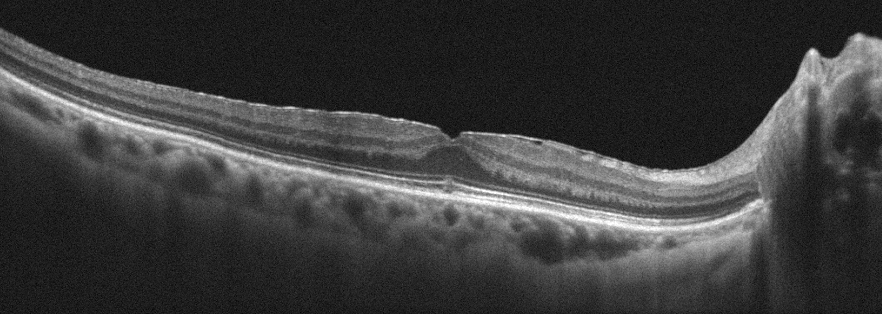
The scan shows ERM.